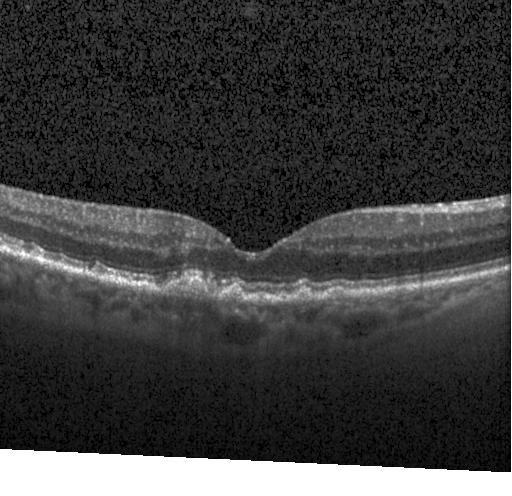 Diagnosis: drusen.